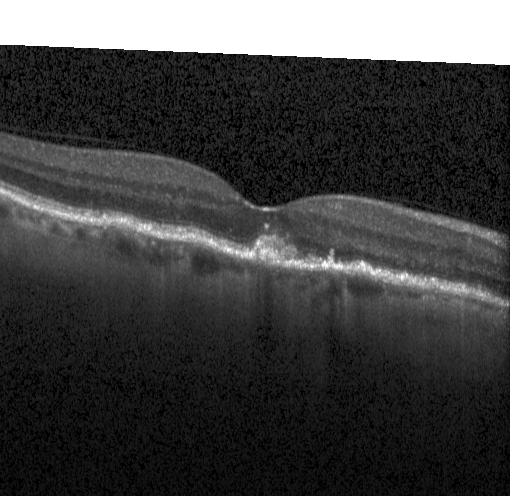
Spectral-domain optical coherence tomography, retinal OCT cross-section. Finding: multiple drusen.